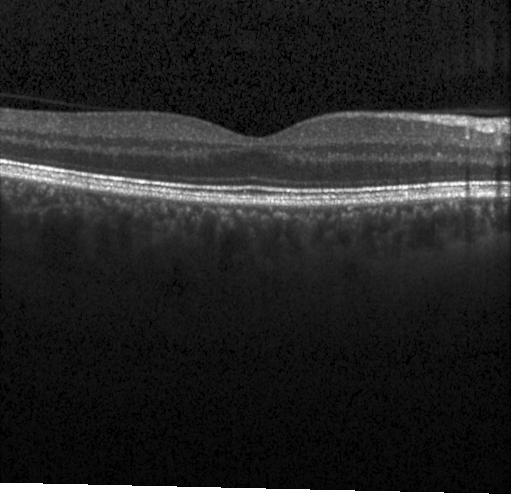

Spectral-domain optical coherence tomography, retinal OCT B-scan
No CNV, DME, or drusen.